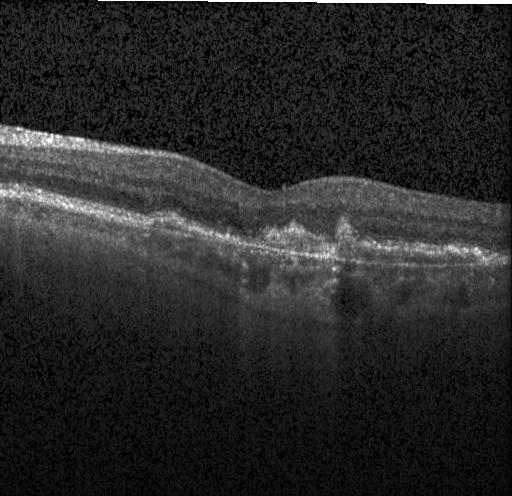 Through the macula. Retinal OCT cross-section. Instrument: Heidelberg Spectralis. Spectral-domain OCT — The scan shows a choroidal neovascular membrane.